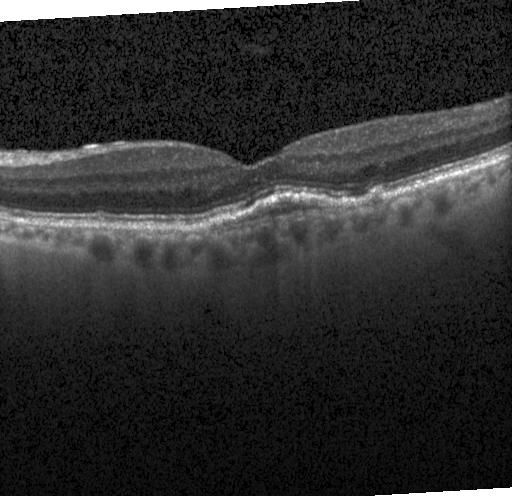 Spectral-domain optical coherence tomography; acquired on a Heidelberg Spectralis; horizontal scan through the fovea; OCT B-scan. Dx: a choroidal neovascular membrane.